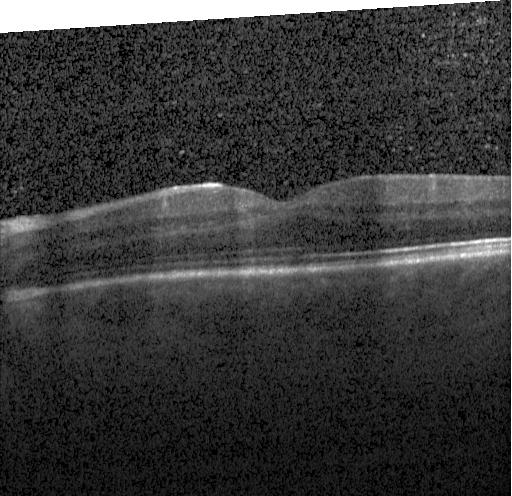
Retinal OCT B-scan · spectral-domain optical coherence tomography · centered on the fovea.
No CNV, no DME, and no drusen.